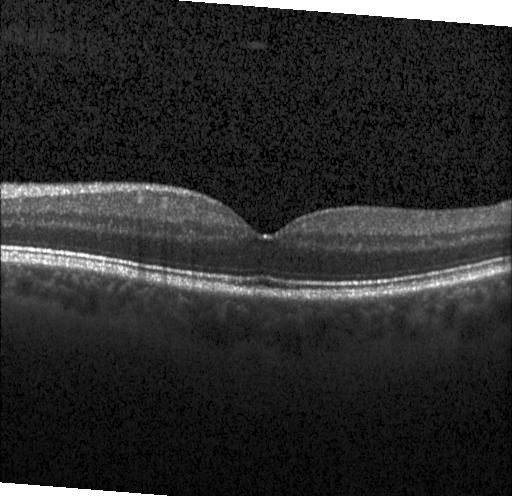
Centered on the fovea · Heidelberg Spectralis OCT system · retinal OCT B-scan · spectral-domain optical coherence tomography. Impression: no evidence of CNV, DME, or drusen.